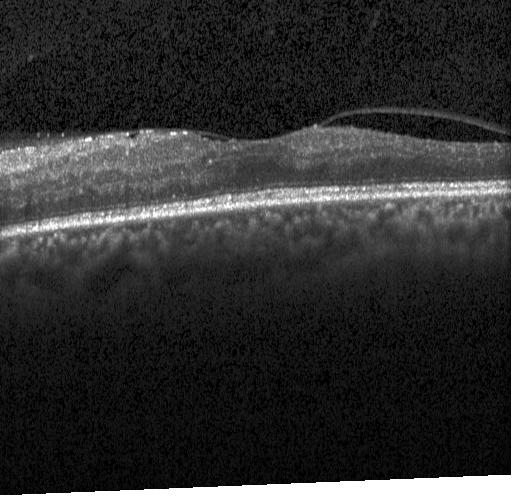
Retinal OCT cross-section — Finding: DME.